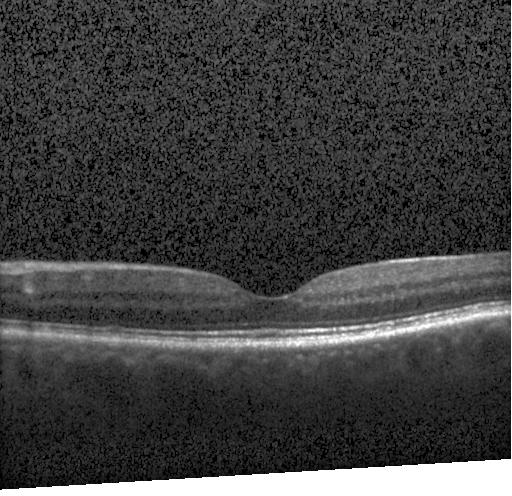 OCT finding: no choroidal neovascularization, diabetic macular edema, or drusen.